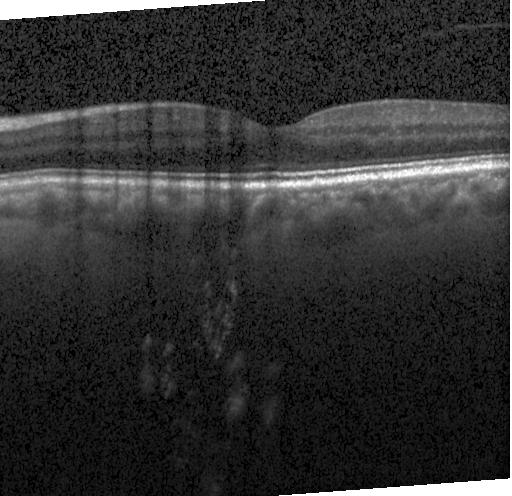
Impression: no choroidal neovascularization, no diabetic macular edema, and no drusen.